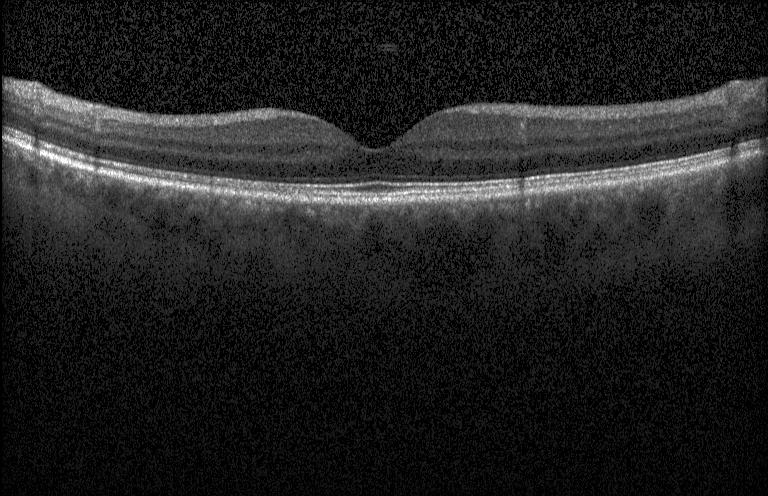

The scan shows neither choroidal neovascularization, diabetic macular edema, nor drusen.